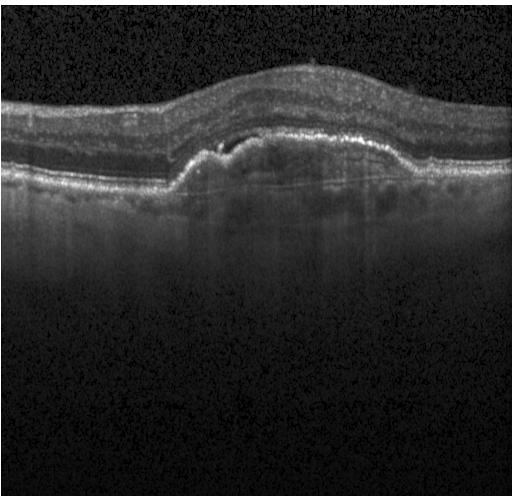
Optical coherence tomography scan; spectral-domain optical coherence tomography.
This B-scan demonstrates a choroidal neovascular membrane.